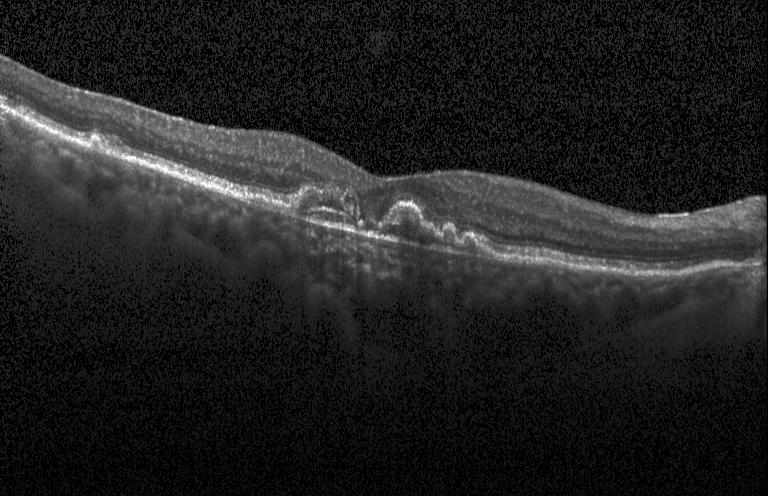

Retinal OCT B-scan
Impression: a choroidal neovascular membrane.